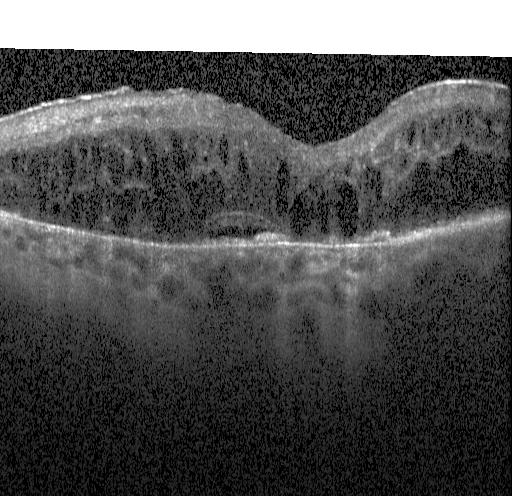
Retinal OCT B-scan. Spectral-domain optical coherence tomography. Instrument: Heidelberg Spectralis.
Impression: a choroidal neovascular membrane.